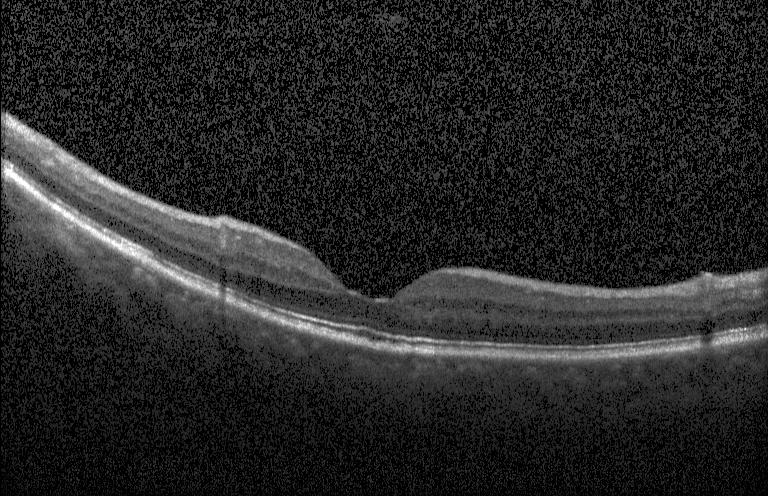 Spectral-domain OCT B-scan: no evidence of choroidal neovascularization, diabetic macular edema, or drusen.